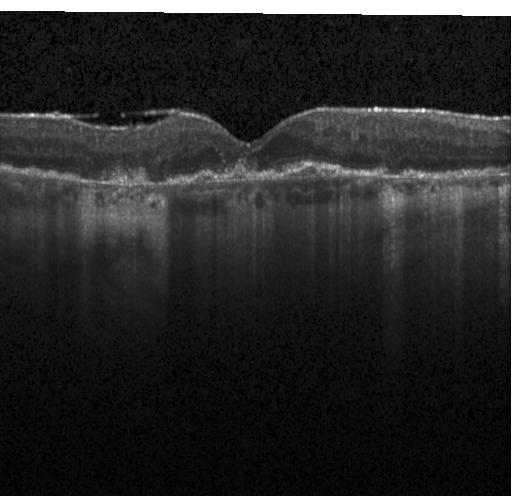

Impression: a choroidal neovascular membrane.